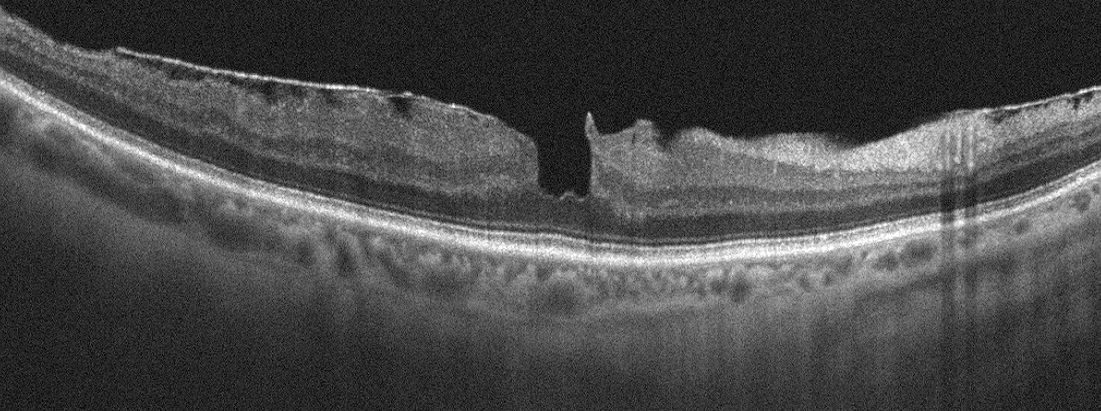

OCT B-scan
Macular OCT: epiretinal membrane (ERM).